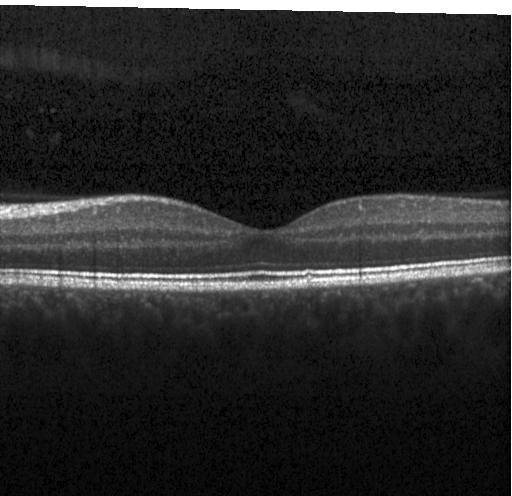 This B-scan demonstrates no choroidal neovascularization, no diabetic macular edema, and no drusen.